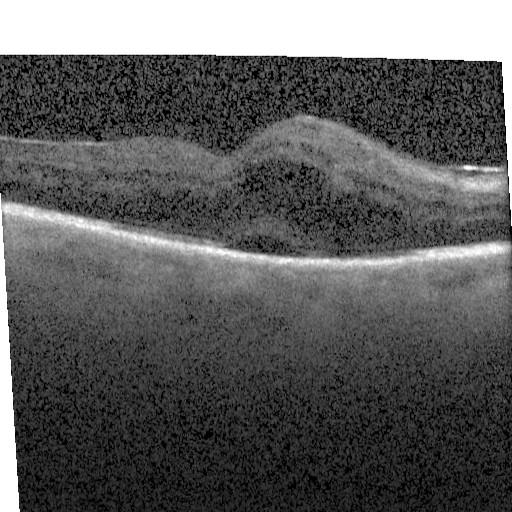
SD-OCT · optical coherence tomography B-scan — Diagnosis: diabetic macular edema.